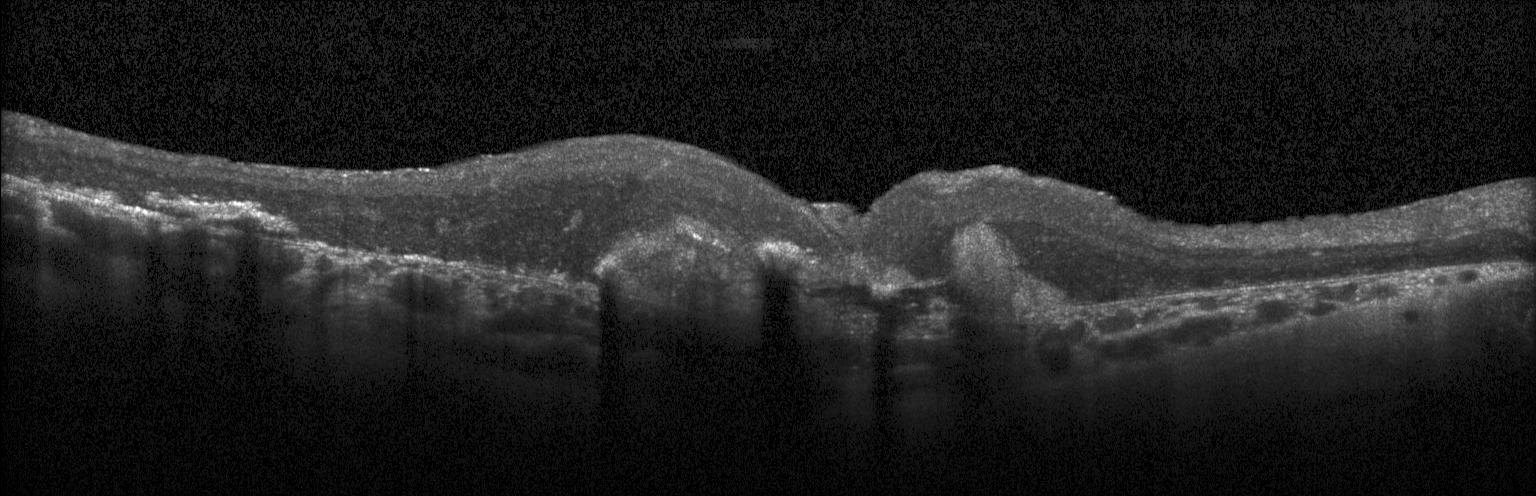 Impression: choroidal neovascularization (CNV).